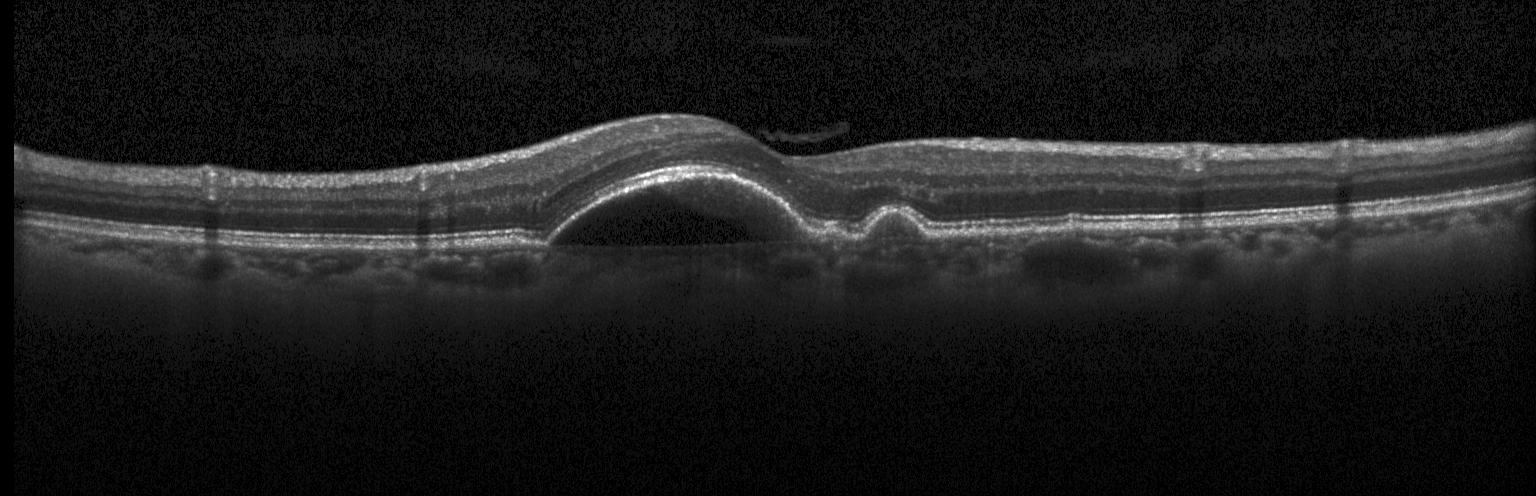 Macular scan, retinal OCT cross-section — Diagnosis: choroidal neovascularization.